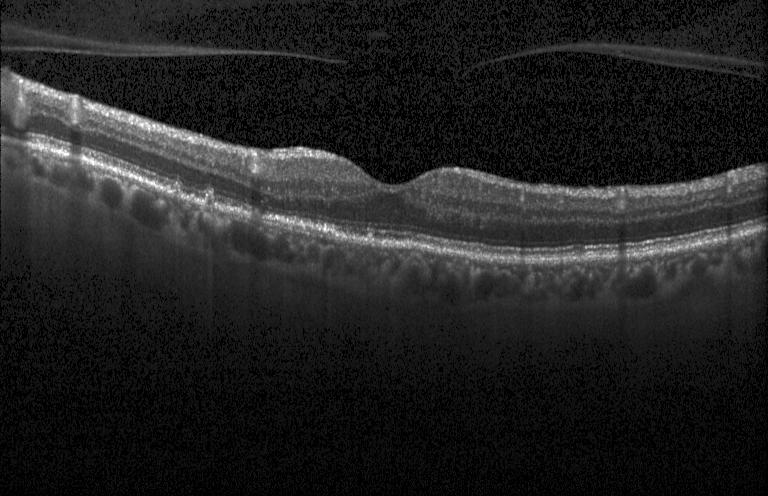 Heidelberg Spectralis OCT system. Centered on the fovea. Optical coherence tomography scan — Impression: drusen.